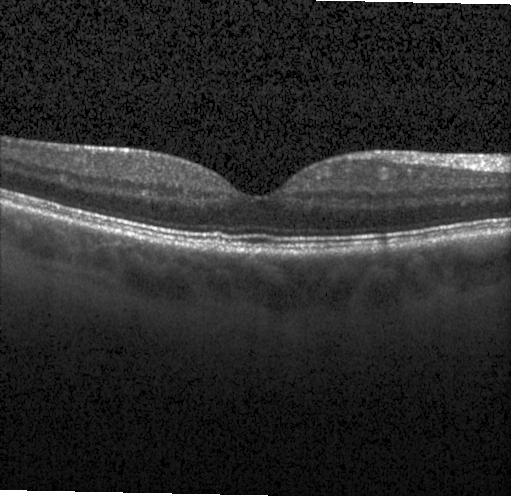 Impression: no CNV, DME, or drusen.